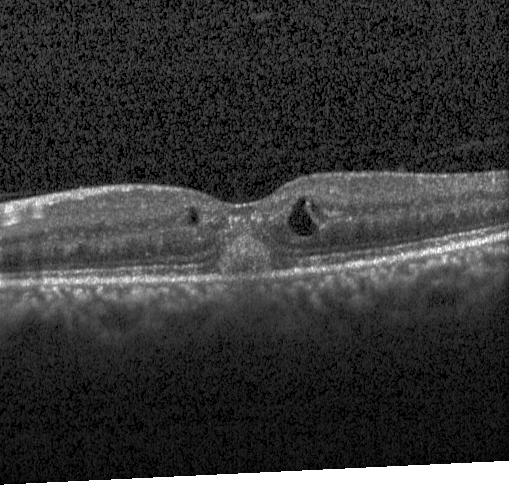

Optical coherence tomography scan, SD-OCT. Dx: CNV.